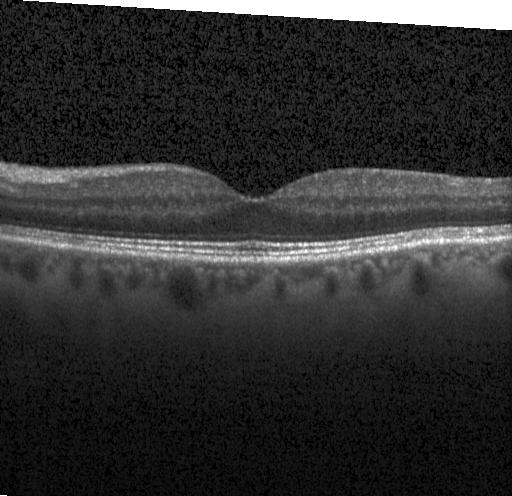
Impression: neither choroidal neovascularization, diabetic macular edema, nor drusen.